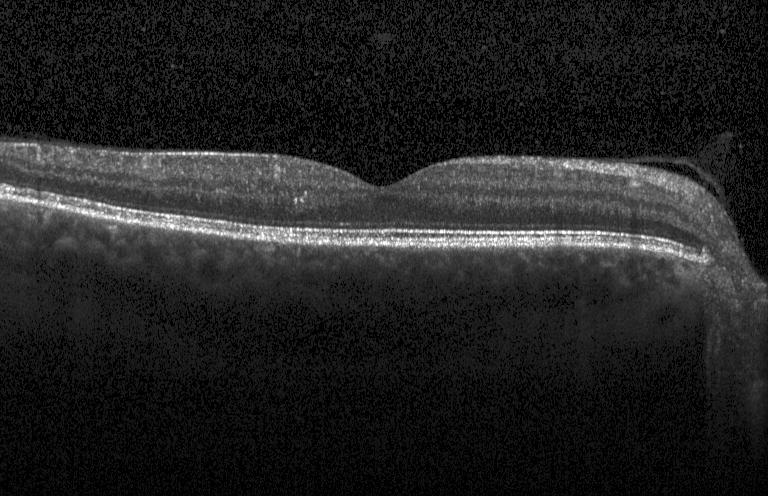

Optical coherence tomography scan. Finding: neither choroidal neovascularization, diabetic macular edema, nor drusen.